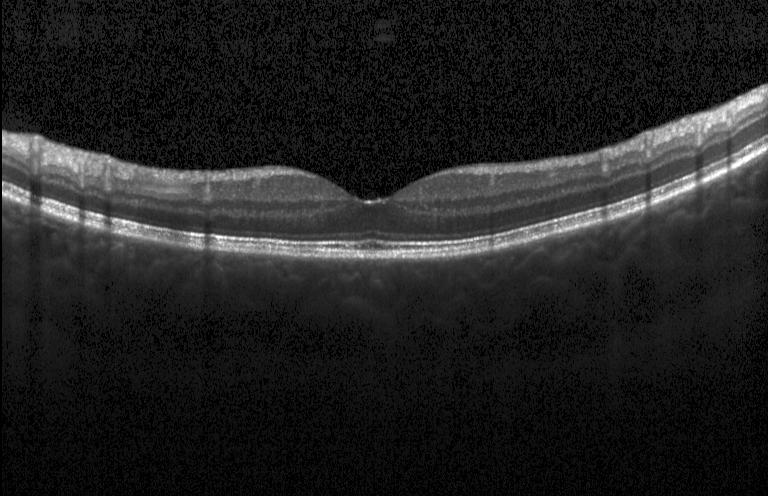 Heidelberg Spectralis OCT system. OCT line scan
Impression: no choroidal neovascularization, diabetic macular edema, or drusen.